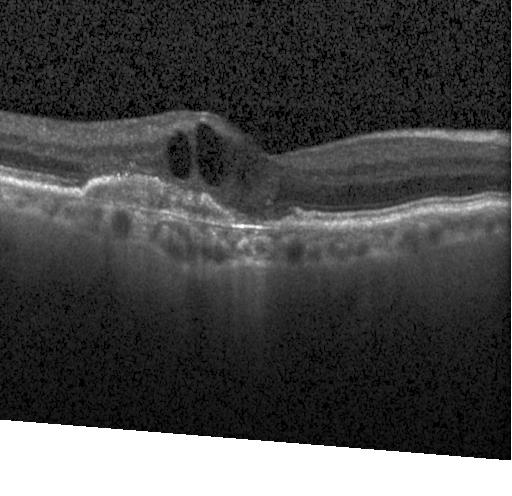
Dx: a choroidal neovascular membrane.